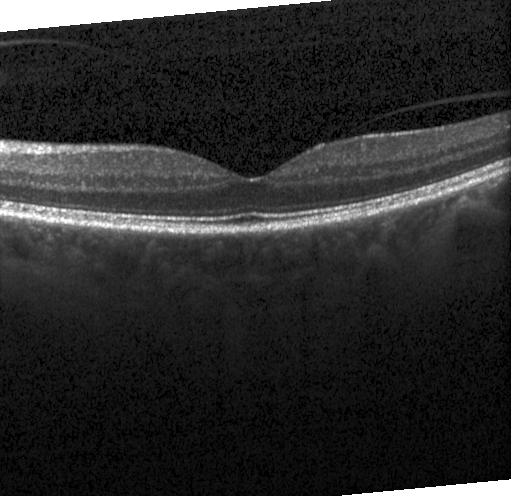
Optical coherence tomography scan, SD-OCT.
Diagnosis: neither CNV, DME, nor drusen.